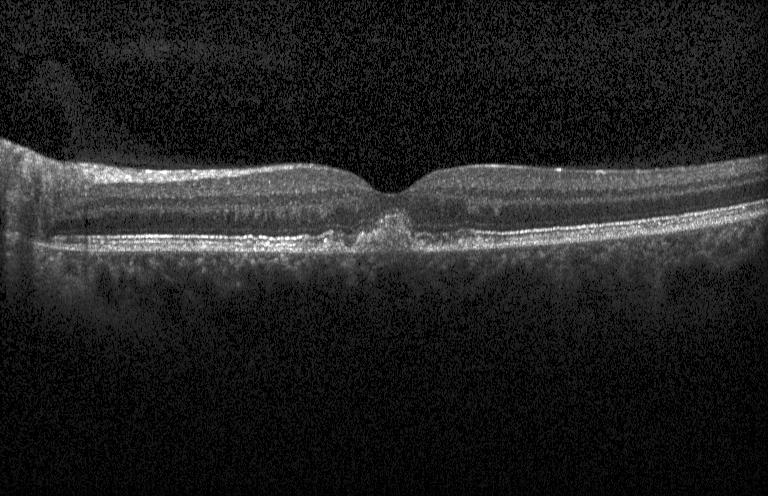
Diagnosis: sub-RPE drusenoid deposits.